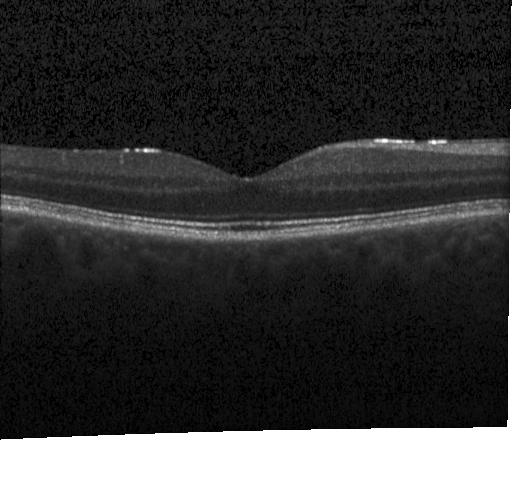
Spectral-domain OCT; retinal OCT cross-section — Impression: neither choroidal neovascularization, diabetic macular edema, nor drusen.